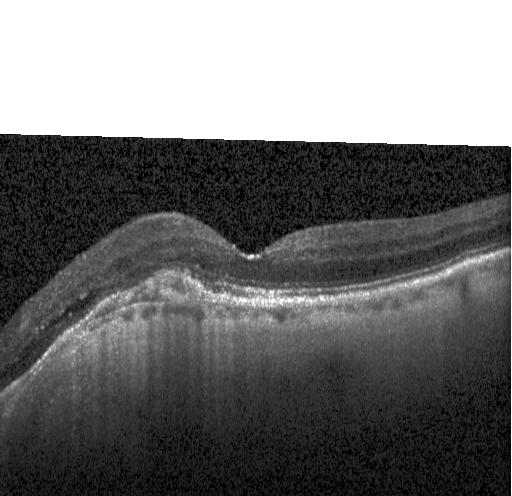
OCT B-scan; macular scan; acquired on a Heidelberg Spectralis.
Diagnosis: a choroidal neovascular membrane.